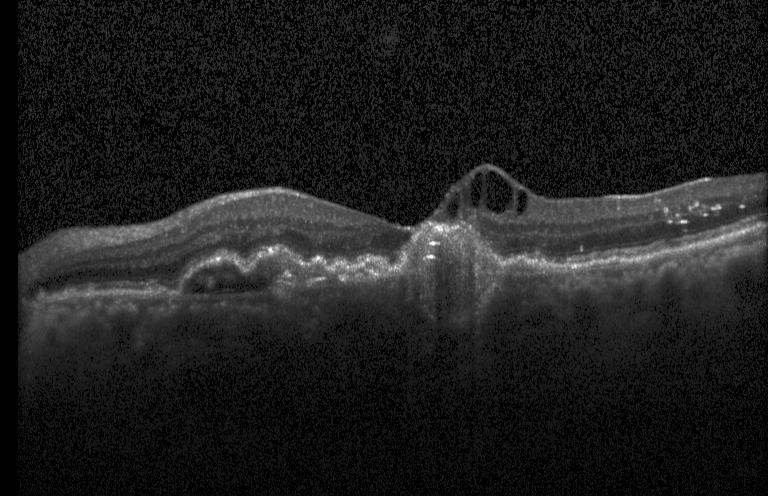

Finding: choroidal neovascularization (CNV).